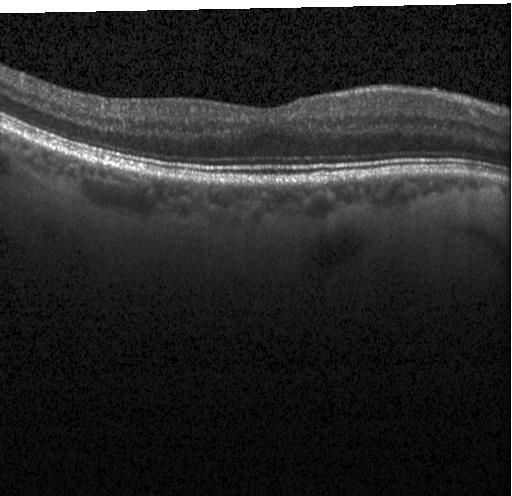

No choroidal neovascularization, no diabetic macular edema, and no drusen.